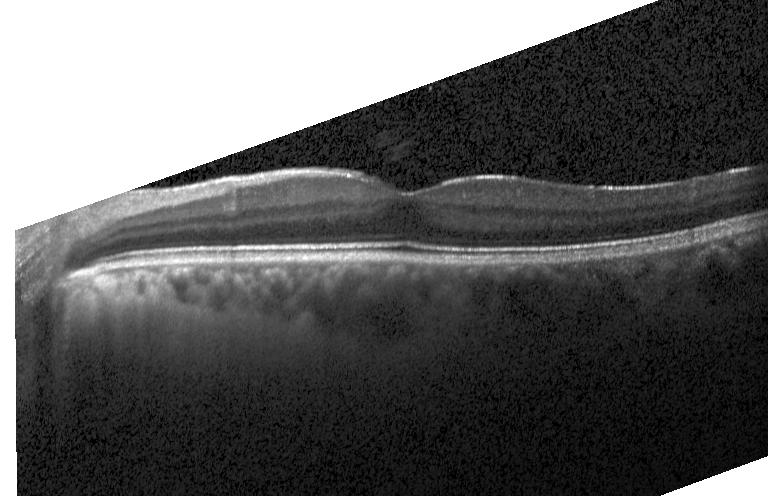

Spectral-domain optical coherence tomography, macular scan, acquired on a Heidelberg Spectralis, OCT B-scan. Diagnosis: neither CNV, DME, nor drusen.